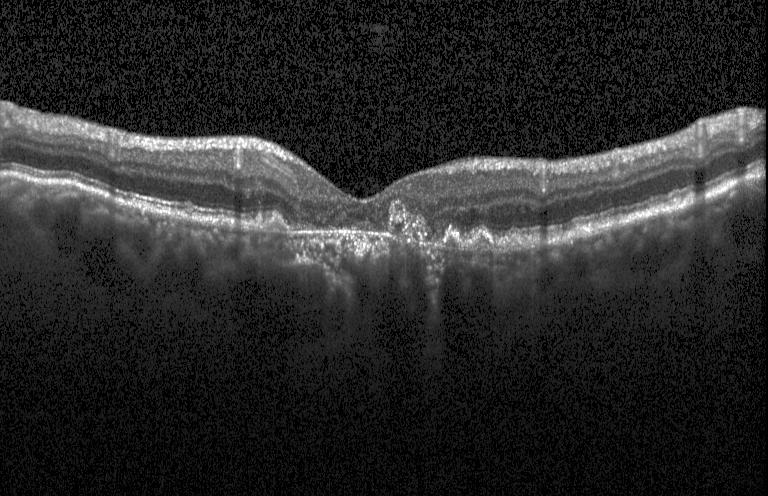

OCT finding: choroidal neovascularization.